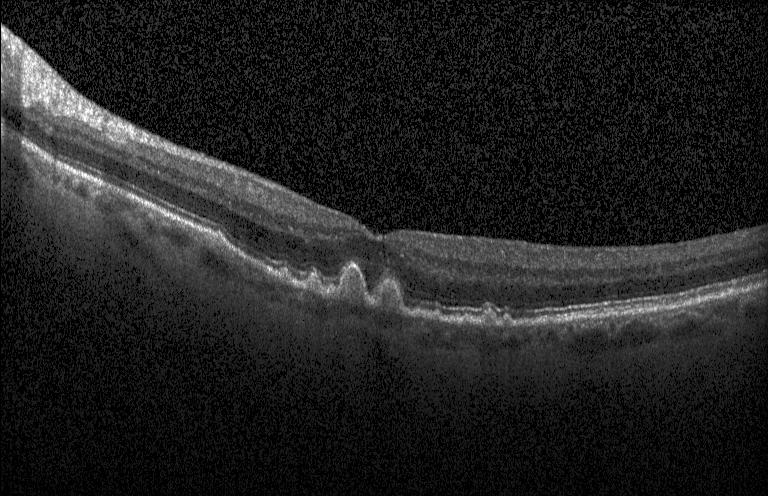

OCT B-scan — Diagnosis: sub-RPE drusenoid deposits.